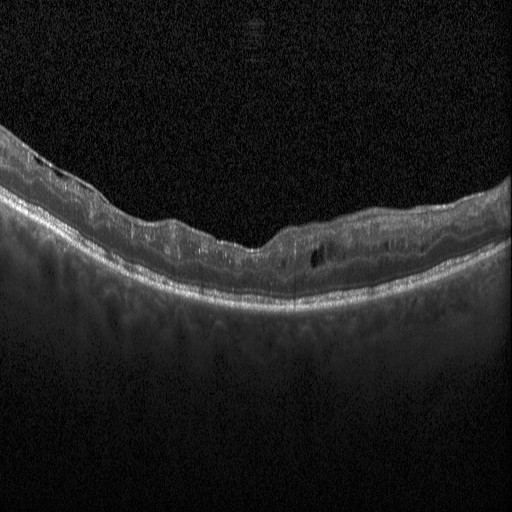

Through the macula. Optical coherence tomography B-scan. Spectral-domain optical coherence tomography. Acquired on a Heidelberg Spectralis.
Impression: DME.